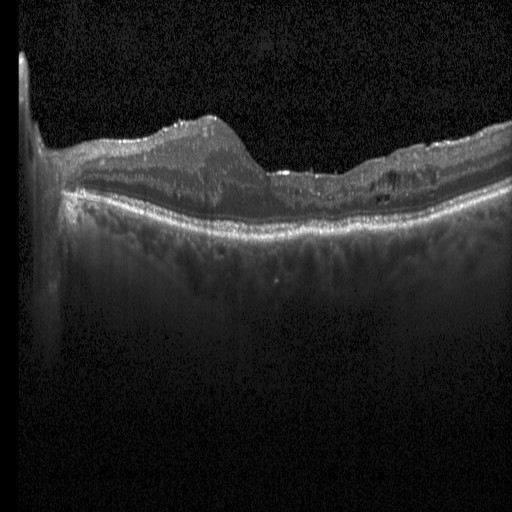 Retinal OCT cross-section showing diabetic macular edema (DME).